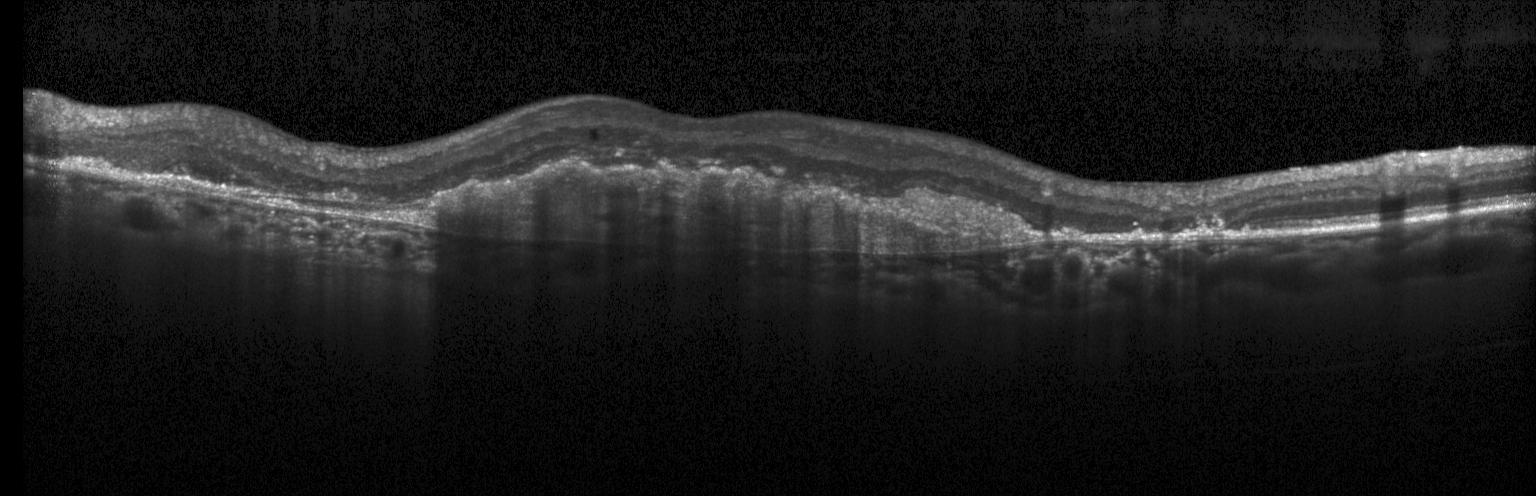
Macular OCT demonstrating CNV.